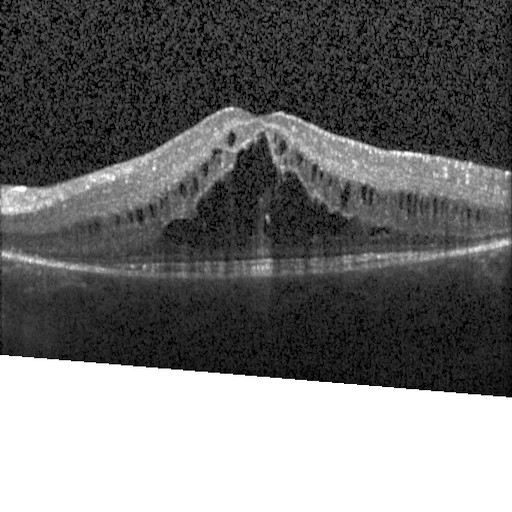

Macular scan, optical coherence tomography scan, SD-OCT, instrument: Heidelberg Spectralis. Assessment: diabetic macular edema.